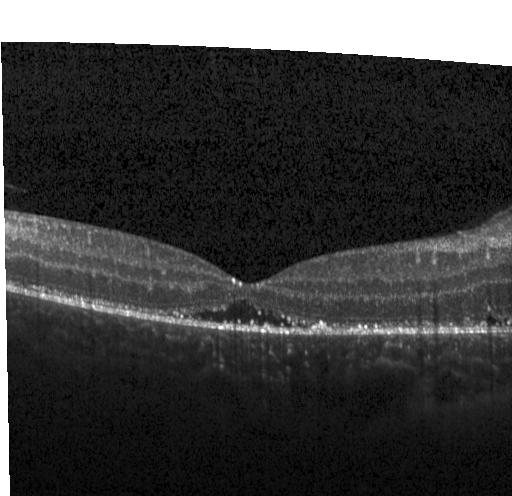
Fovea-centered. Instrument: Heidelberg Spectralis. Retinal OCT cross-section.
Diagnosis: choroidal neovascularization.